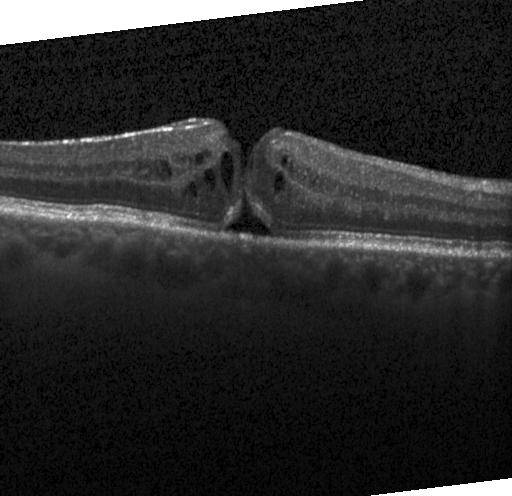 Optical coherence tomography scan — Diagnosis: diabetic macular edema.